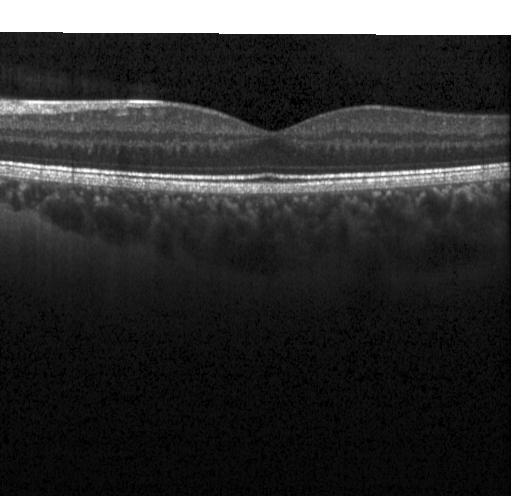 Spectral-domain optical coherence tomography; fovea-centered; optical coherence tomography B-scan.
Finding: no evidence of CNV, DME, or drusen.